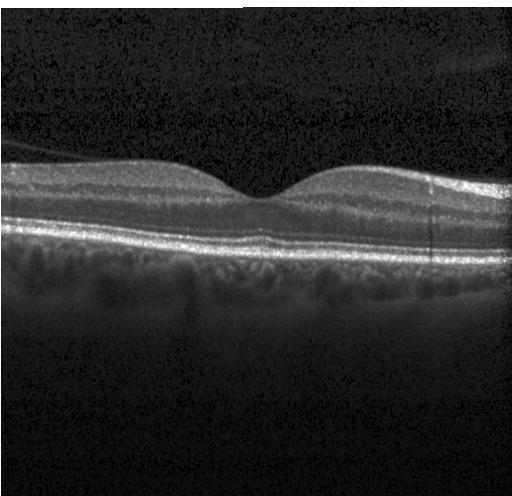
OCT scan showing no choroidal neovascularization, diabetic macular edema, or drusen.